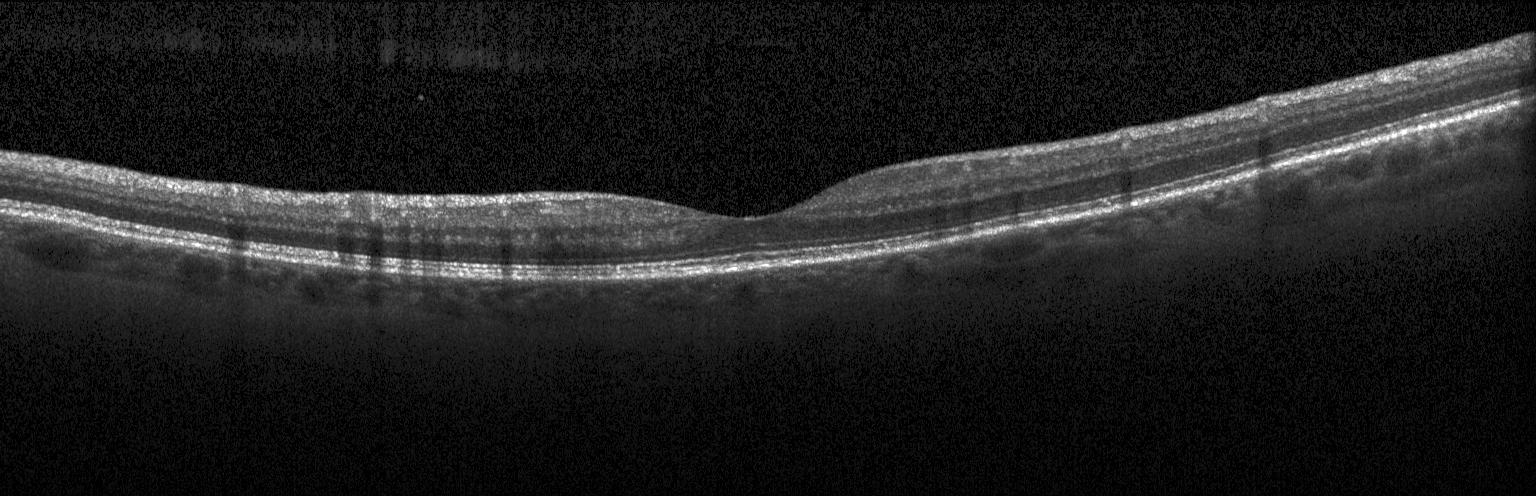 Macular OCT demonstrating neither CNV, DME, nor drusen.